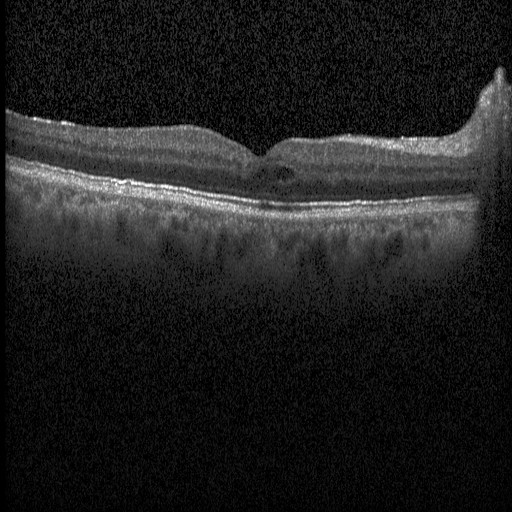 Horizontal scan through the fovea; retinal OCT B-scan
This B-scan demonstrates diabetic macular edema (DME).